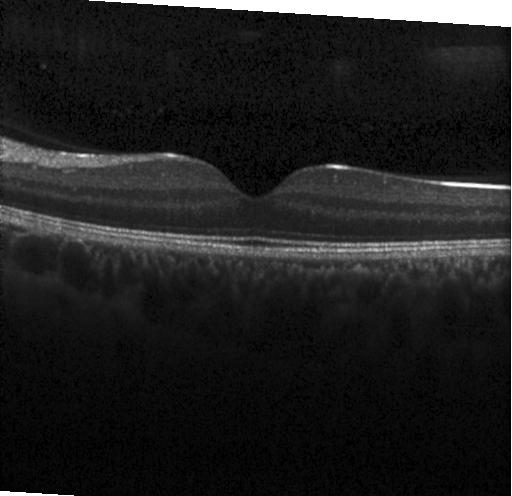
Spectral-domain optical coherence tomography · Heidelberg Spectralis · retinal OCT cross-section · through the macula
This B-scan demonstrates no evidence of choroidal neovascularization, diabetic macular edema, or drusen.